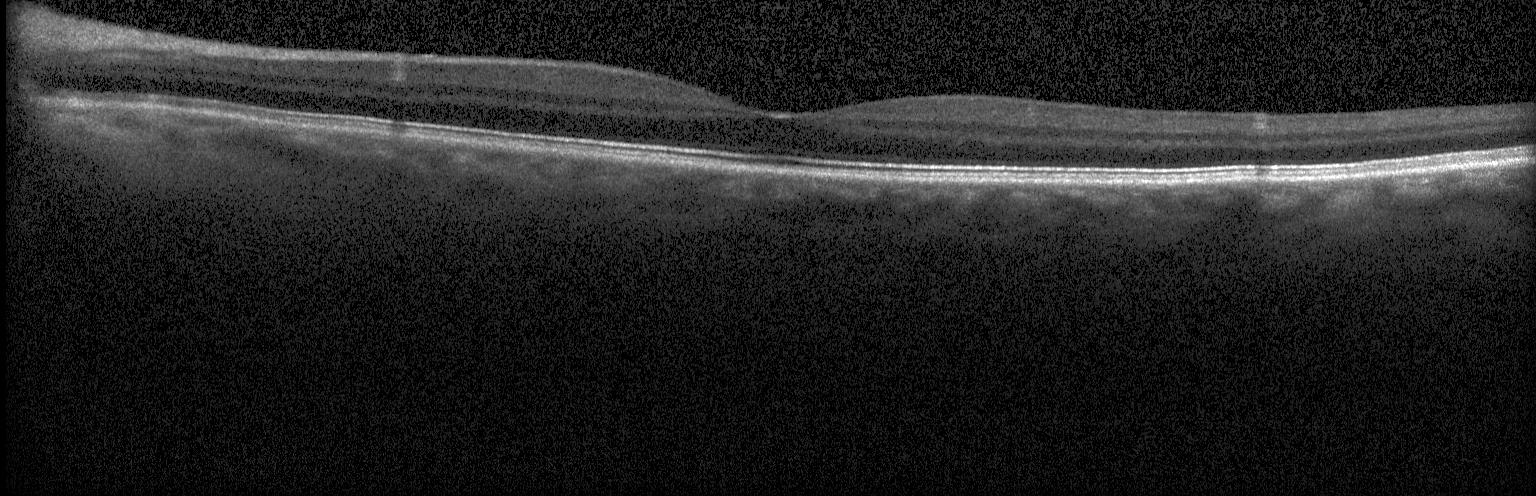
Heidelberg Spectralis OCT system, retinal OCT cross-section. OCT finding: no choroidal neovascularization, no diabetic macular edema, and no drusen.